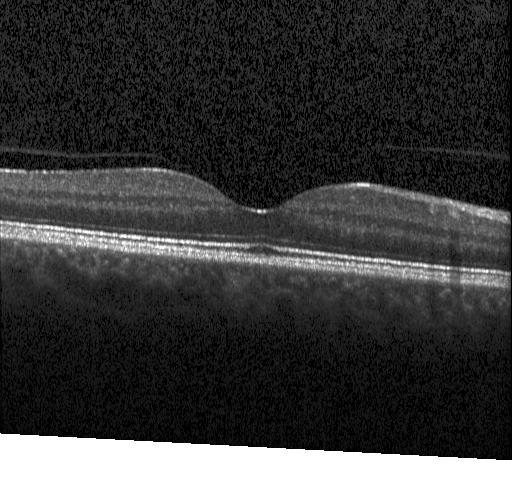
Assessment: neither choroidal neovascularization, diabetic macular edema, nor drusen.